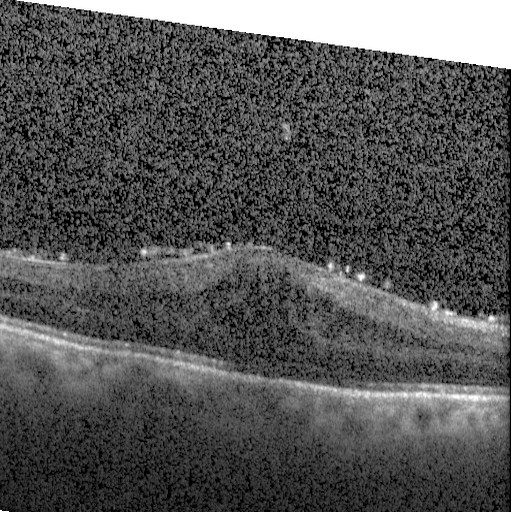 Optical coherence tomography B-scan
This B-scan demonstrates diabetic macular edema.